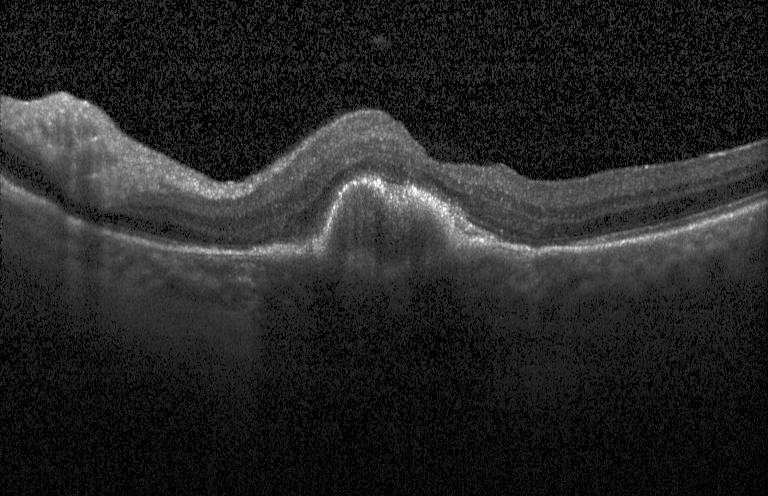
Heidelberg Spectralis. Centered on the fovea. Retinal OCT cross-section. SD-OCT. Dx: a choroidal neovascular membrane.